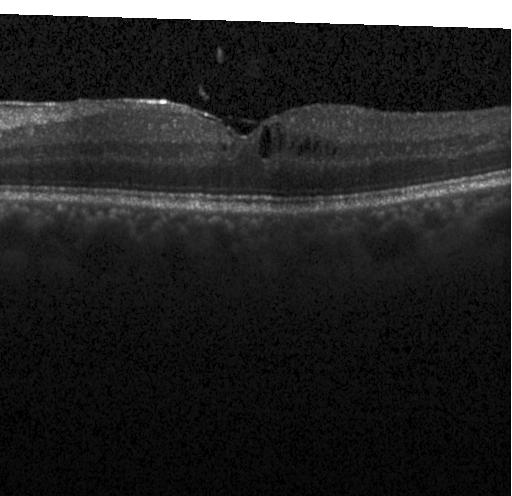
OCT scan showing diabetic macular edema (DME).